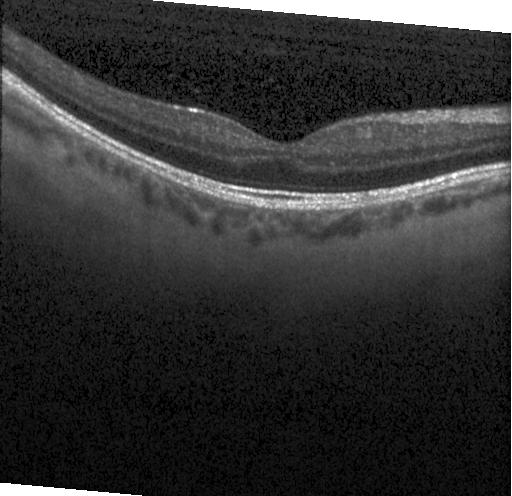
Centered on the fovea; Heidelberg Spectralis OCT system; optical coherence tomography scan.
Dx: no choroidal neovascularization, no diabetic macular edema, and no drusen.